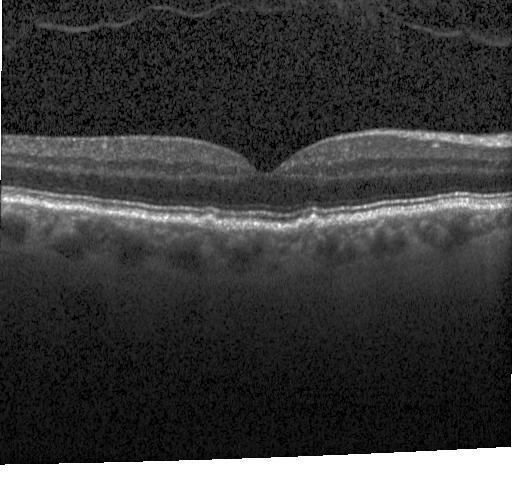
Macular OCT demonstrating drusen.